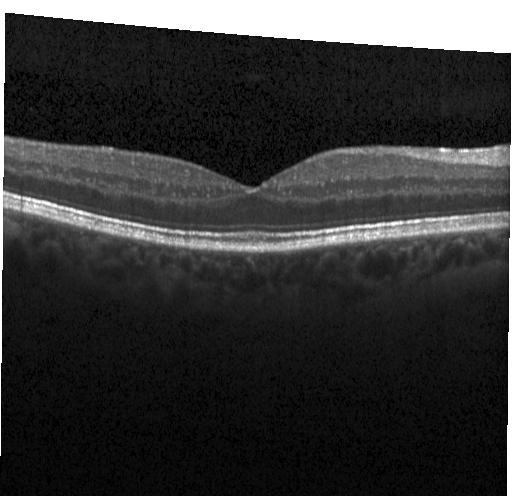
Diagnosis: no CNV, DME, or drusen.